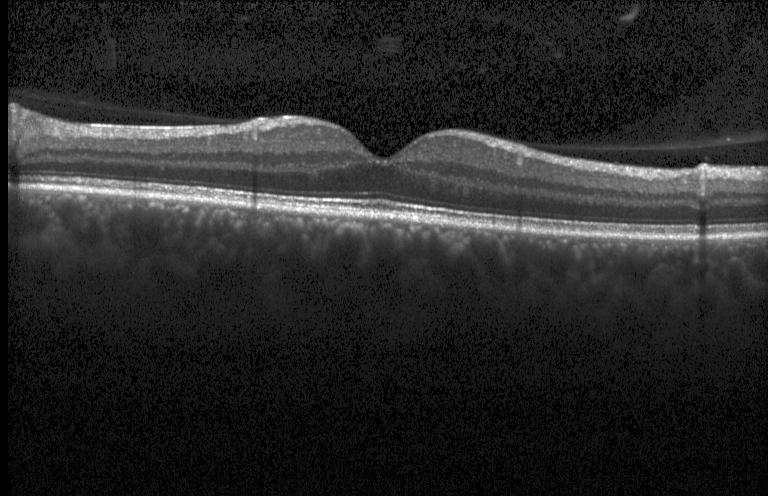
Optical coherence tomography scan. Impression: neither choroidal neovascularization, diabetic macular edema, nor drusen.